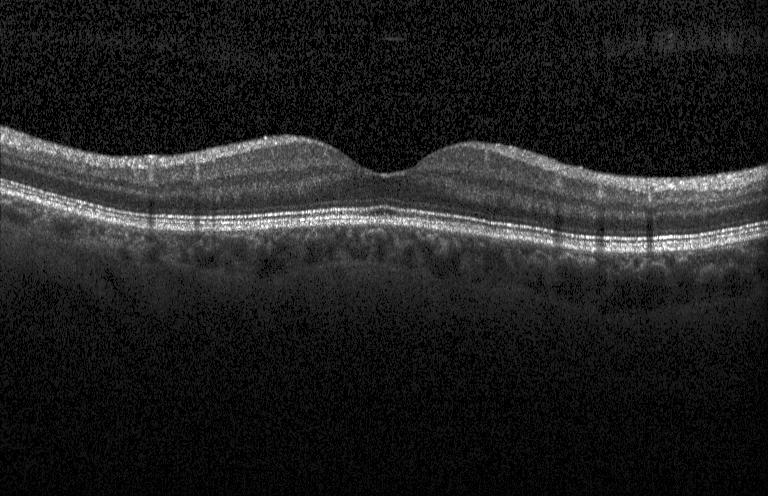

Impression: no evidence of choroidal neovascularization, diabetic macular edema, or drusen.